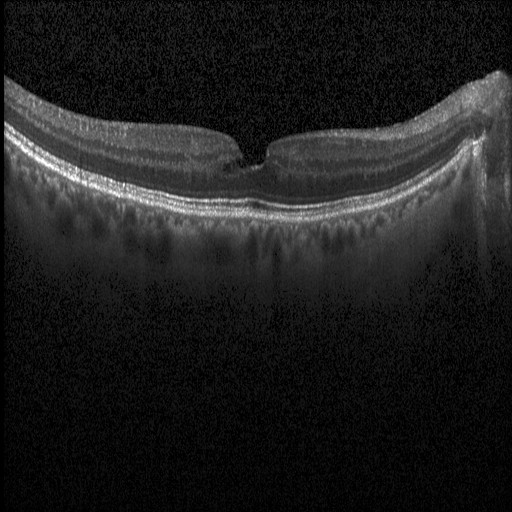 Optical coherence tomography B-scan.
Impression: diabetic macular edema (DME).